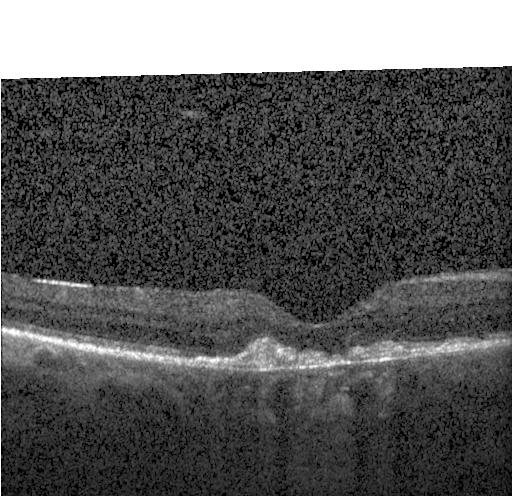

Instrument: Heidelberg Spectralis · SD-OCT · optical coherence tomography scan · through the macula.
Choroidal neovascularization (CNV).